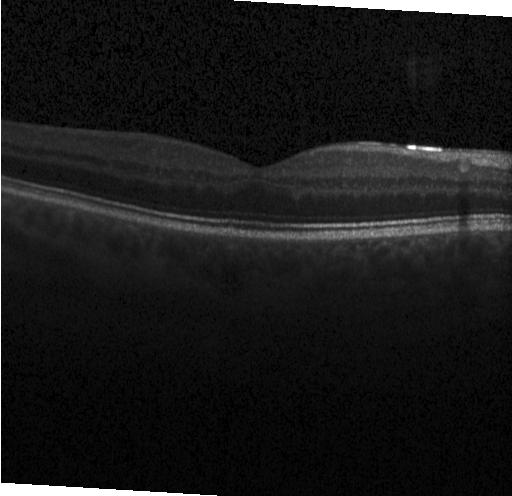

Diagnosis: no evidence of CNV, DME, or drusen.